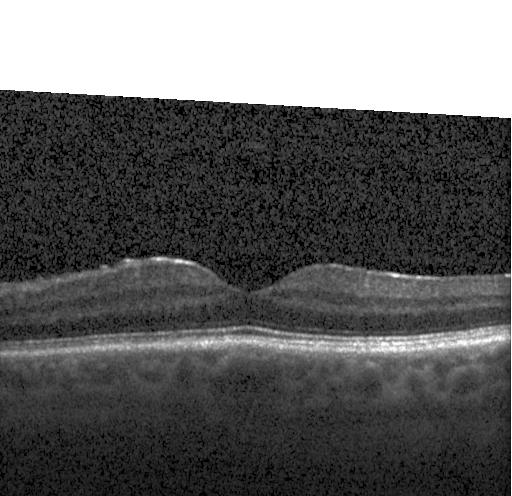 Optical coherence tomography scan. OCT finding: no CNV, DME, or drusen.